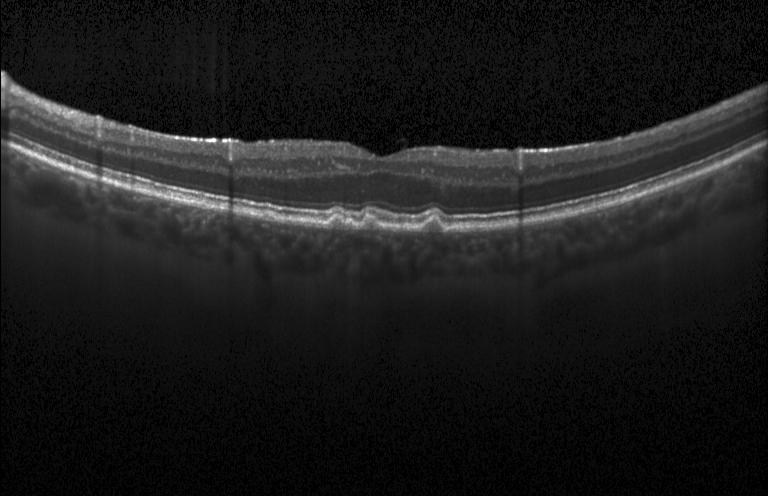 Optical coherence tomography scan
Macular OCT: drusen.